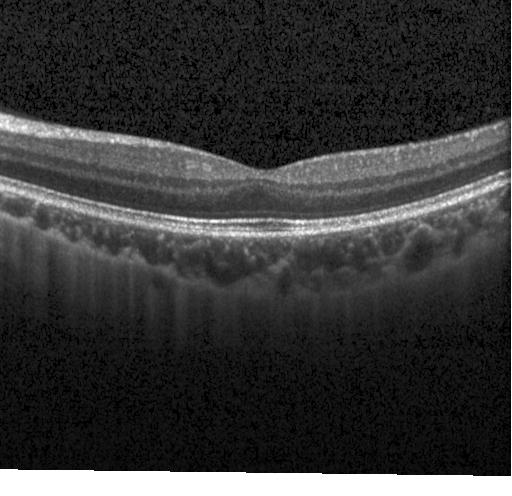 Impression: neither choroidal neovascularization, diabetic macular edema, nor drusen.